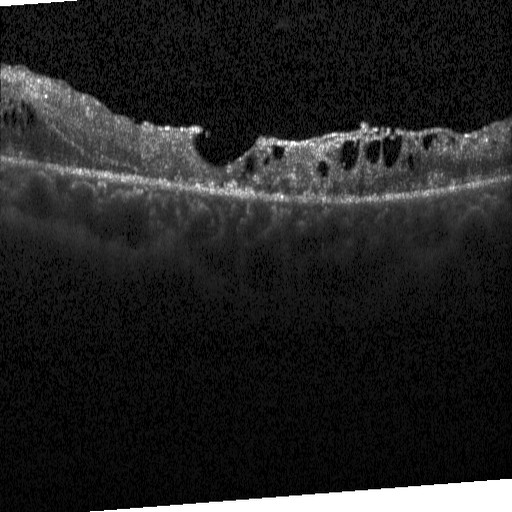 Retinal OCT cross-section. Diagnosis: diabetic macular edema.